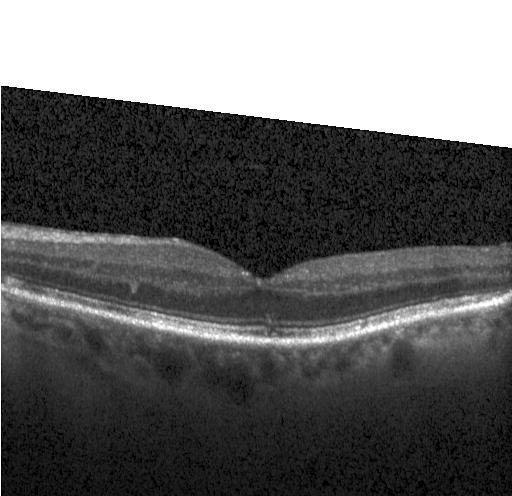
OCT B-scan showing no choroidal neovascularization, no diabetic macular edema, and no drusen.